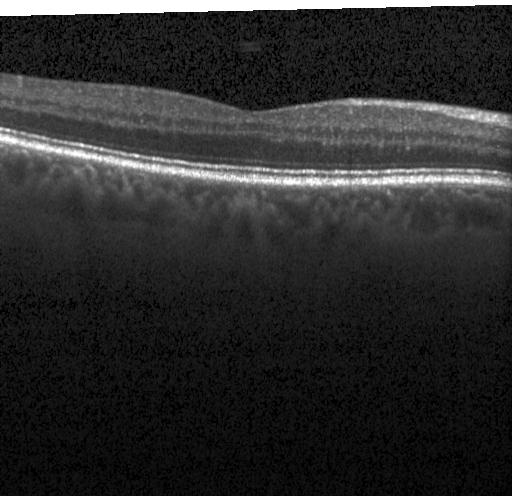 Optical coherence tomography scan. Diagnosis: no CNV, DME, or drusen.